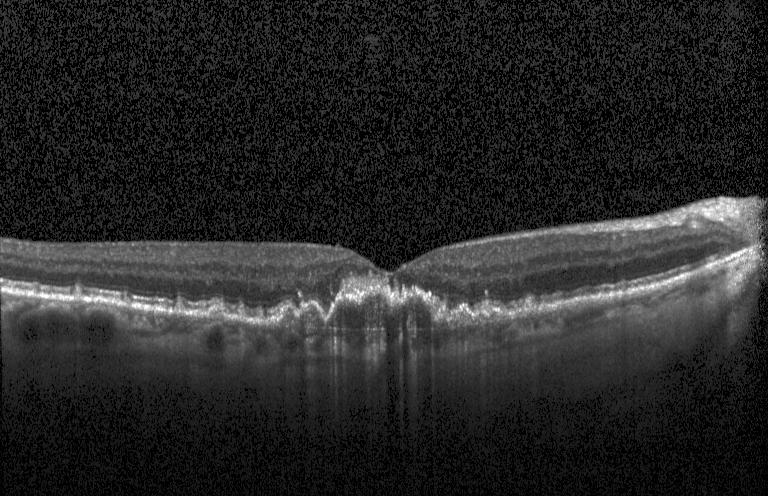
Diagnosis: a choroidal neovascular membrane.